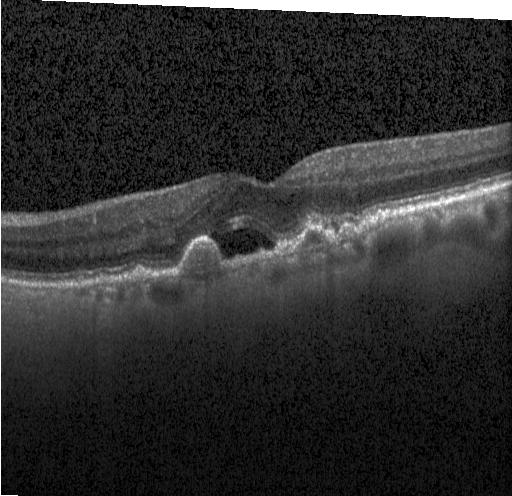

Optical coherence tomography B-scan
Dx: a choroidal neovascular membrane.